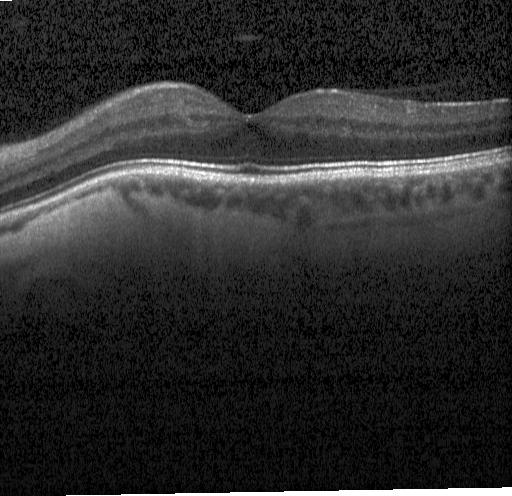

Optical coherence tomography scan. SD-OCT. Heidelberg Spectralis OCT system — Impression: no CNV, DME, or drusen.